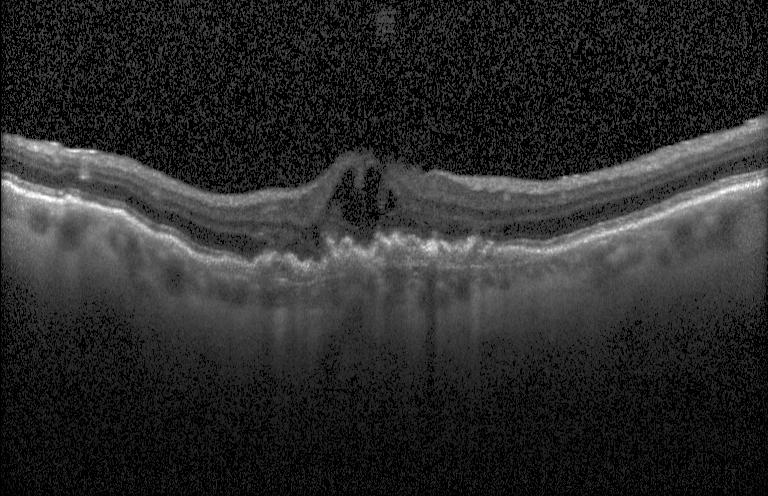

OCT B-scan. Through the macula. Macular OCT: a choroidal neovascular membrane.